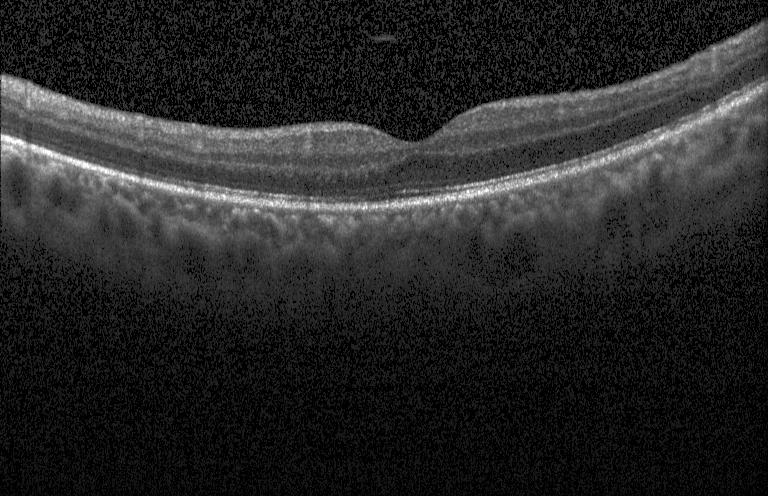

OCT B-scan · instrument: Heidelberg Spectralis · fovea-centered · SD-OCT — Diagnosis: no evidence of CNV, DME, or drusen.